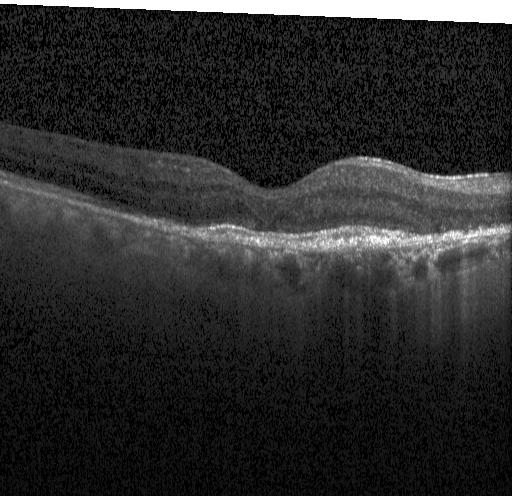 Centered on the fovea, optical coherence tomography scan, spectral-domain OCT — The scan shows a choroidal neovascular membrane.